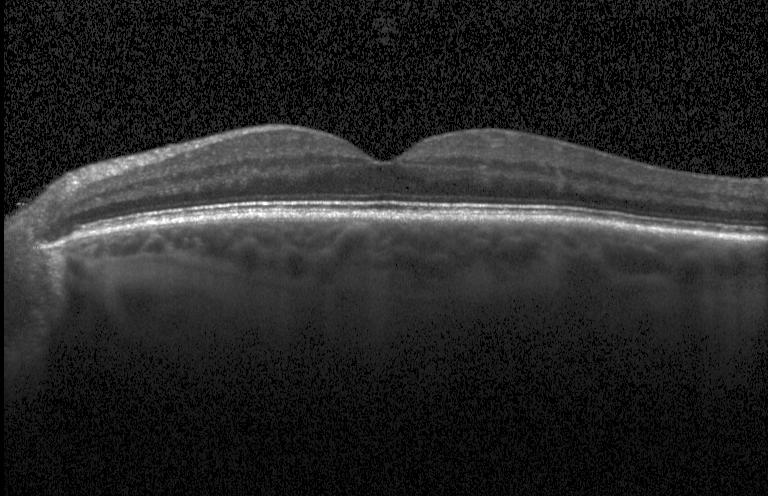

OCT B-scan.
OCT finding: neither choroidal neovascularization, diabetic macular edema, nor drusen.